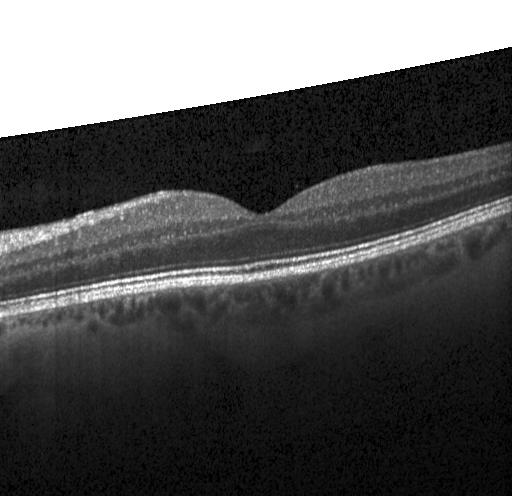
Fovea-centered; OCT line scan. Finding: no evidence of CNV, DME, or drusen.